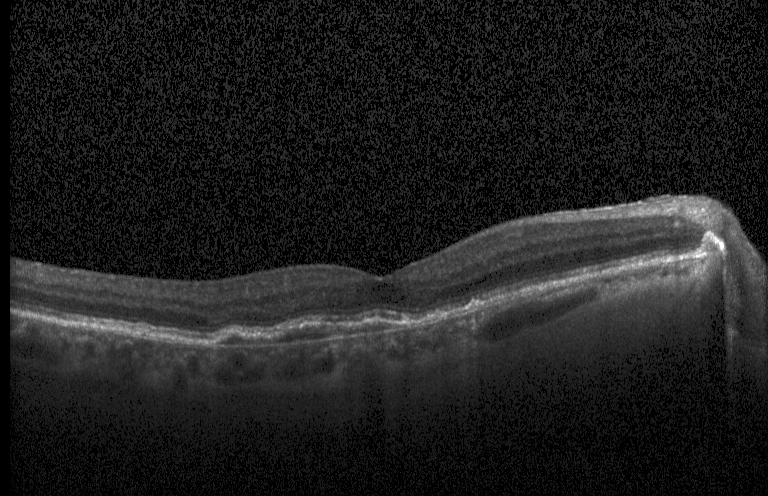 Retinal OCT B-scan. Finding: choroidal neovascularization.